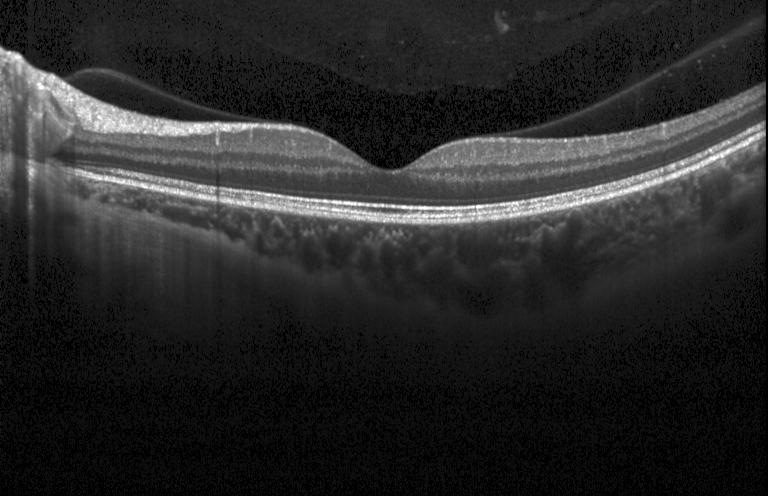

Macular OCT: neither choroidal neovascularization, diabetic macular edema, nor drusen.